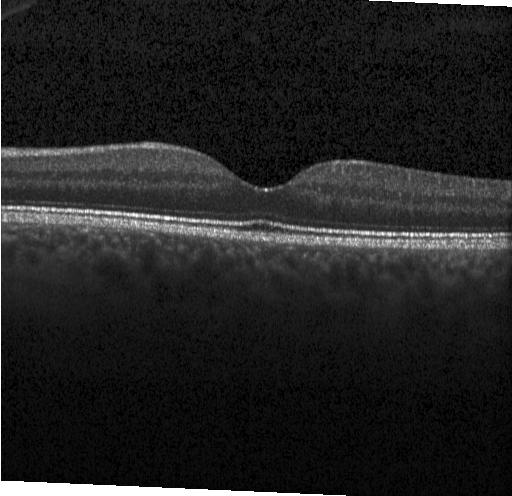 Retinal OCT cross-section; horizontal scan through the fovea — Finding: no evidence of CNV, DME, or drusen.